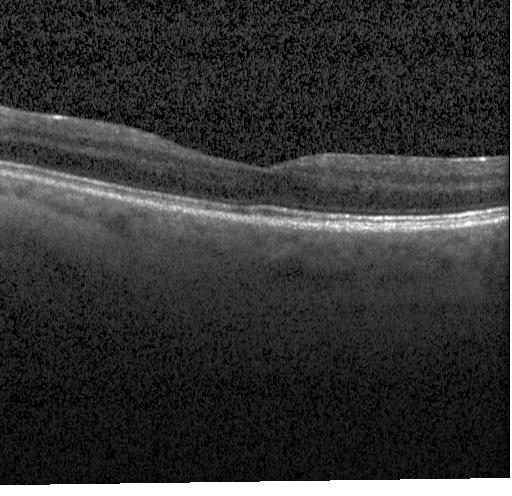 SD-OCT; retinal OCT B-scan.
Diagnosis: neither choroidal neovascularization, diabetic macular edema, nor drusen.